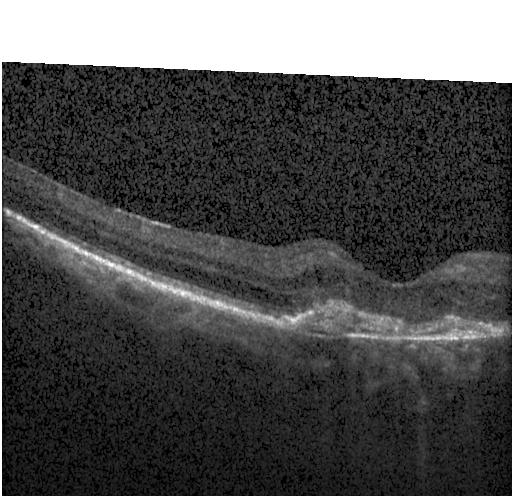 Assessment: choroidal neovascularization (CNV).